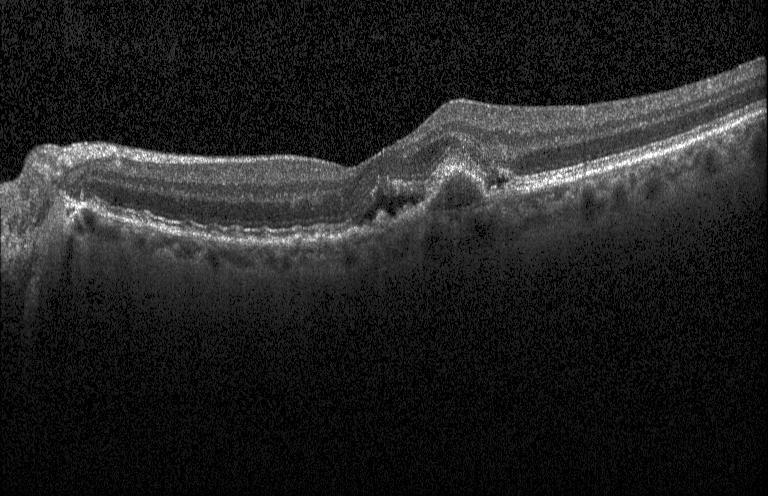

OCT line scan · SD-OCT
Diagnosis: a choroidal neovascular membrane.